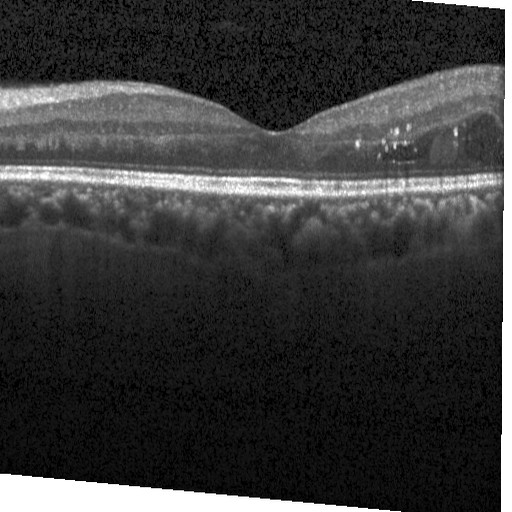

Macular OCT demonstrating diabetic macular edema (DME).